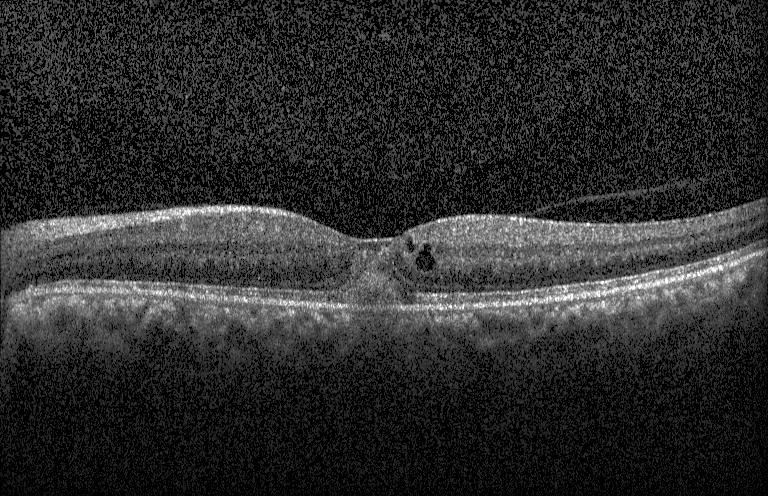
OCT line scan, centered on the fovea, SD-OCT, instrument: Heidelberg Spectralis. Impression: choroidal neovascularization (CNV).